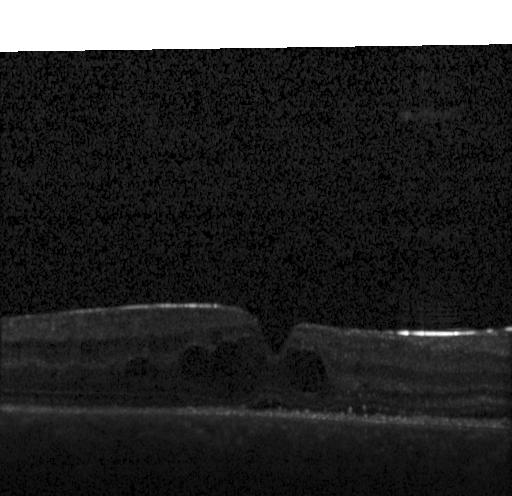 Macular OCT: DME.